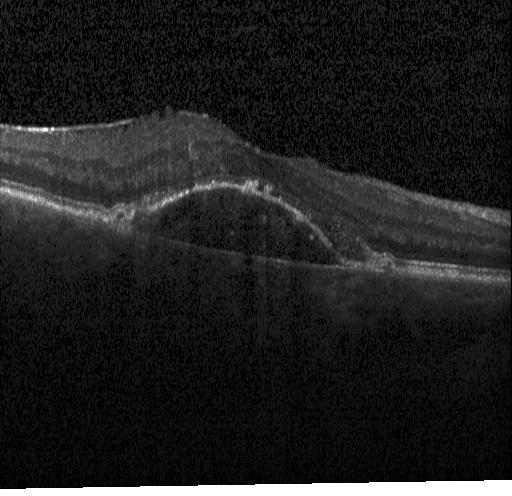

Impression: a choroidal neovascular membrane.